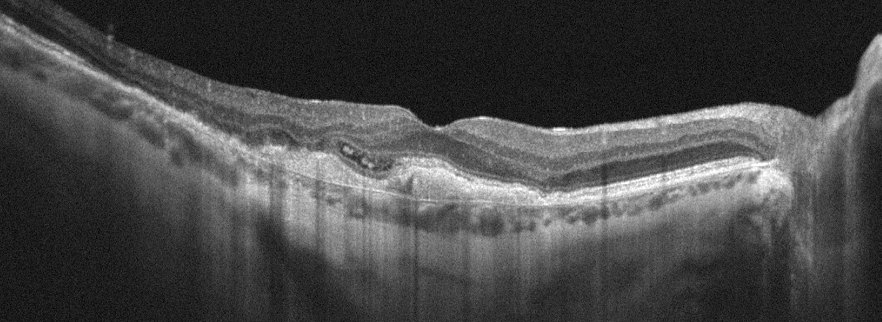

Oculus dexter, optical coherence tomography scan. Age-related macular degeneration.